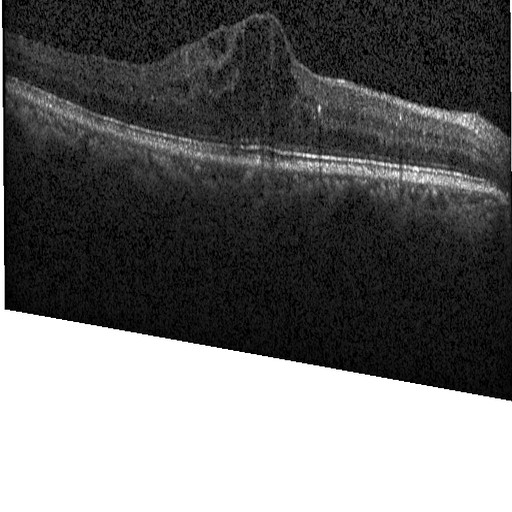
The scan shows DME.